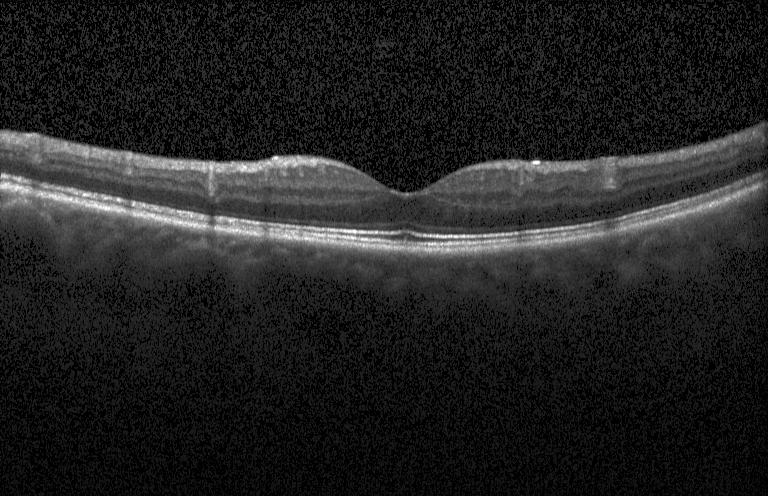 Optical coherence tomography B-scan, horizontal scan through the fovea — Dx: no choroidal neovascularization, diabetic macular edema, or drusen.